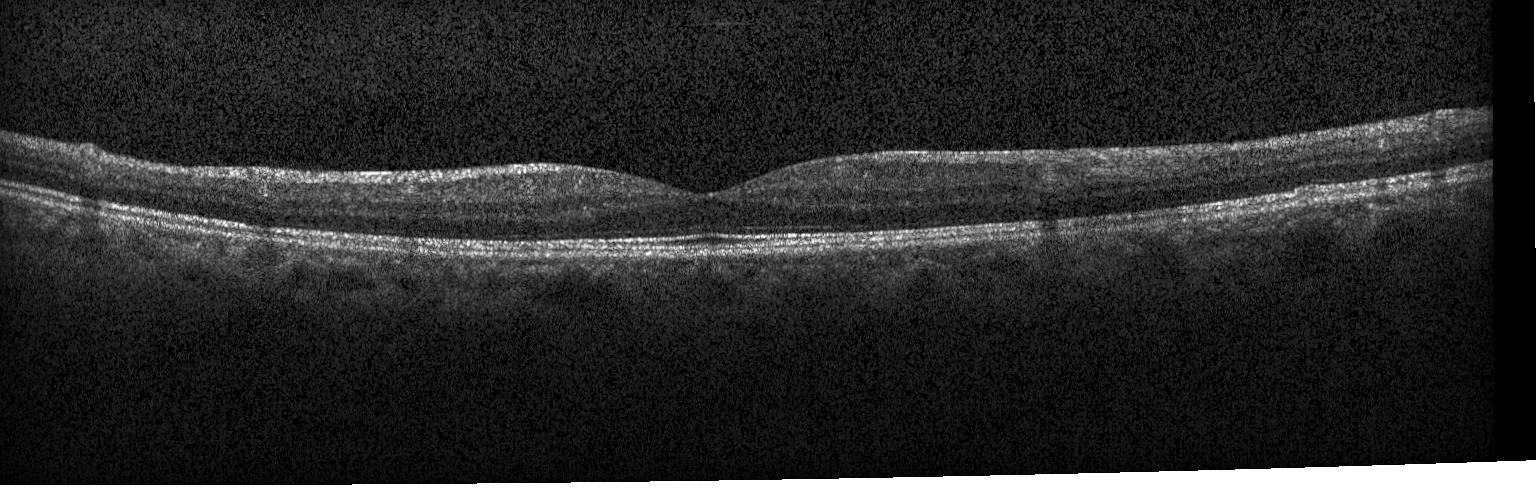

Optical coherence tomography B-scan.
Assessment: no choroidal neovascularization, no diabetic macular edema, and no drusen.